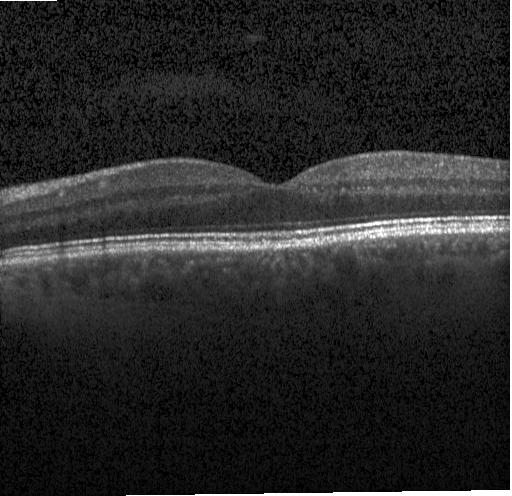
Impression: no choroidal neovascularization, no diabetic macular edema, and no drusen.